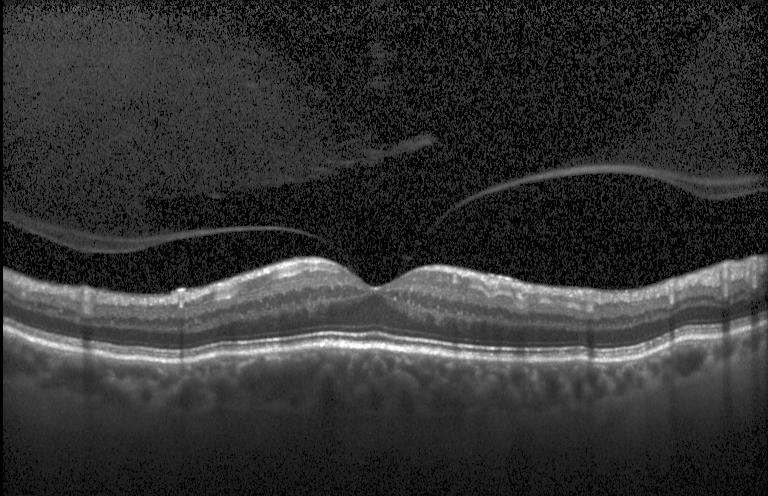
Fovea-centered; spectral-domain optical coherence tomography; optical coherence tomography B-scan — Impression: no choroidal neovascularization, diabetic macular edema, or drusen.